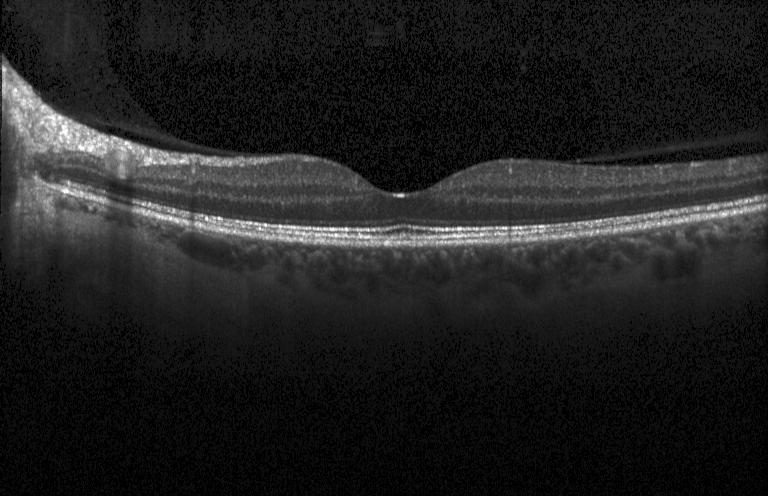 Optical coherence tomography scan; through the macula; acquired on a Heidelberg Spectralis; spectral-domain optical coherence tomography — Impression: no choroidal neovascularization, diabetic macular edema, or drusen.